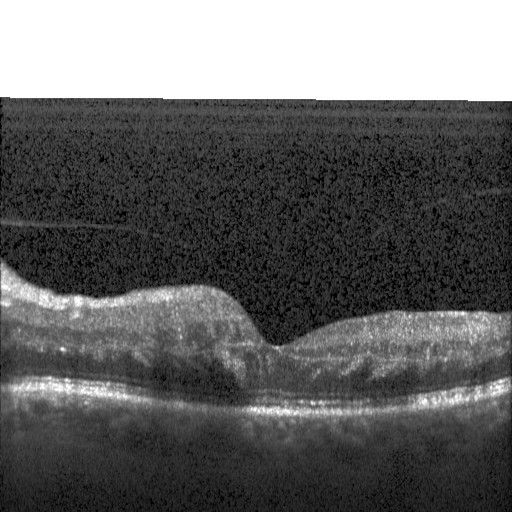
Diabetic macular edema (DME).